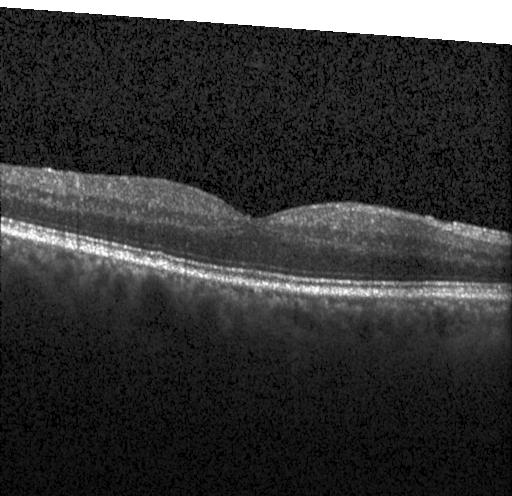 Retinal OCT cross-section showing neither choroidal neovascularization, diabetic macular edema, nor drusen.